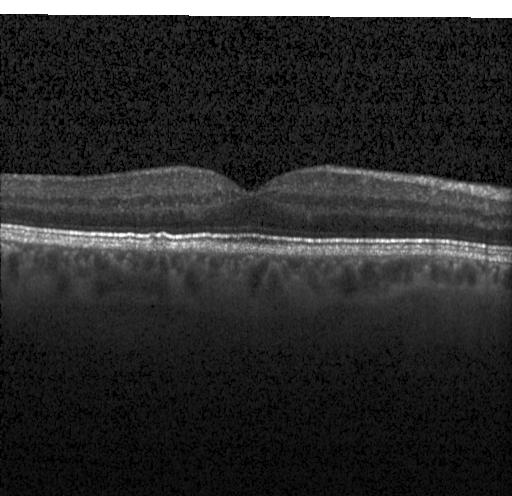
Horizontal scan through the fovea, Heidelberg Spectralis OCT system, retinal OCT B-scan, SD-OCT.
Multiple drusen.